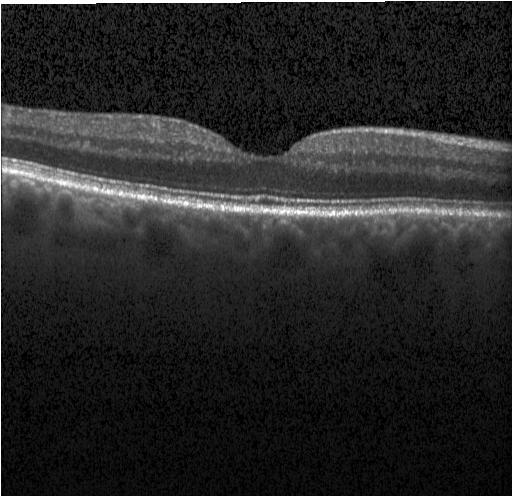
Diagnosis: no choroidal neovascularization, diabetic macular edema, or drusen.